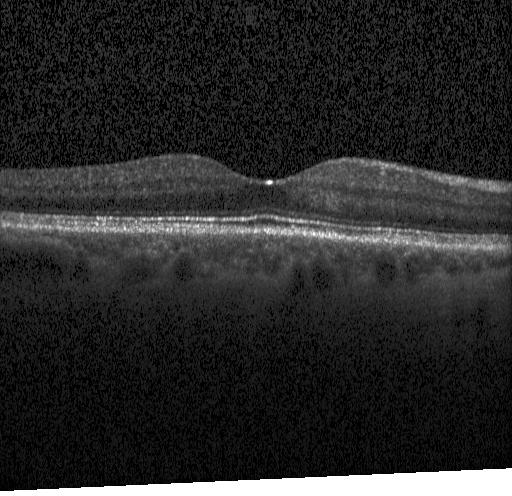
Optical coherence tomography scan; centered on the fovea — Impression: no evidence of choroidal neovascularization, diabetic macular edema, or drusen.